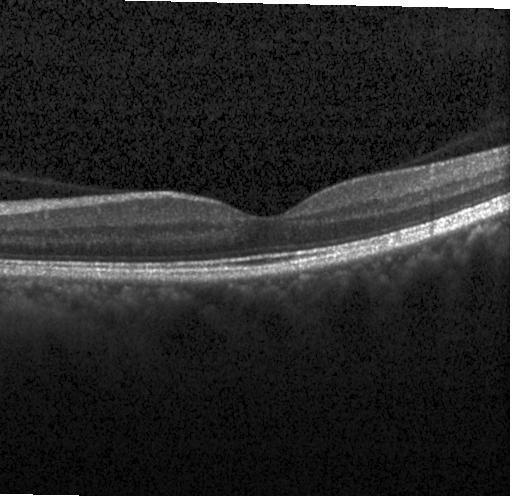

Heidelberg Spectralis OCT system; retinal OCT B-scan; fovea-centered — Assessment: no CNV, no DME, and no drusen.